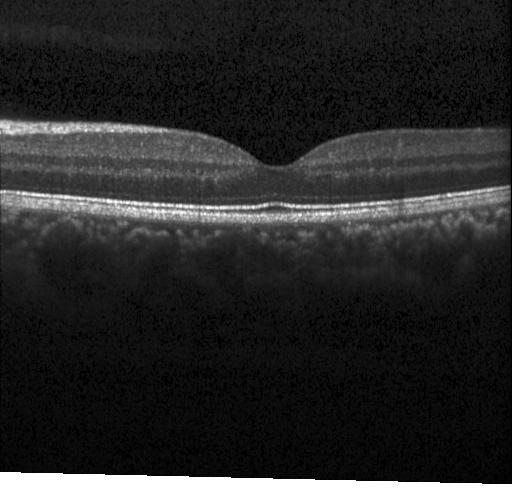 Macular OCT demonstrating no choroidal neovascularization, no diabetic macular edema, and no drusen.